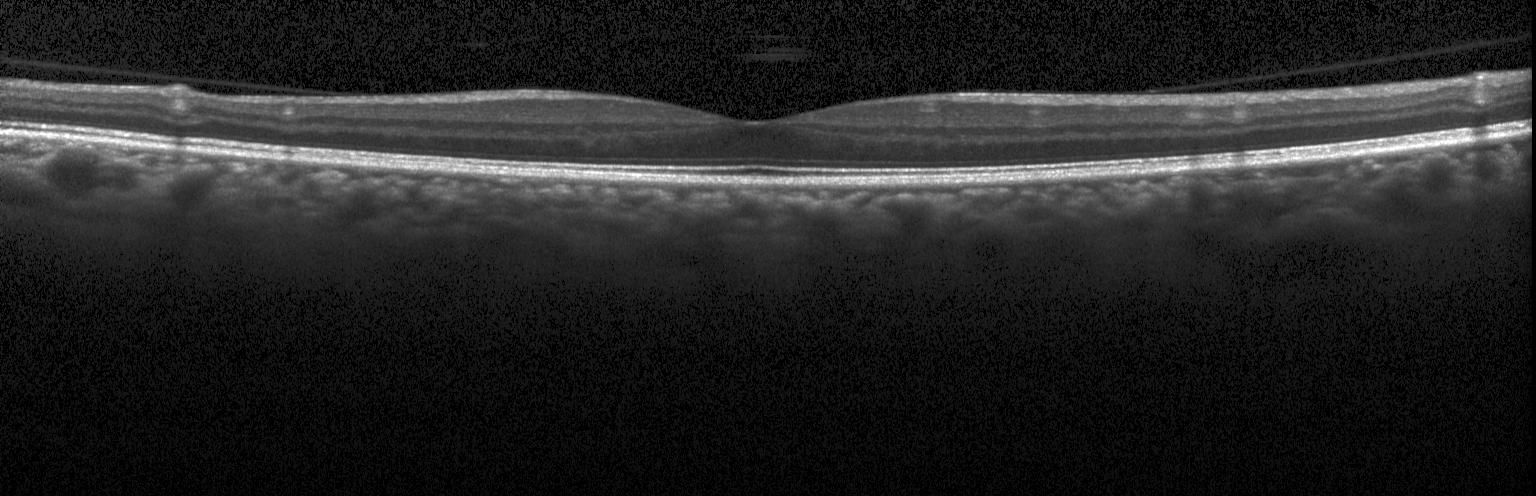 Retinal OCT B-scan — Impression: no CNV, no DME, and no drusen.